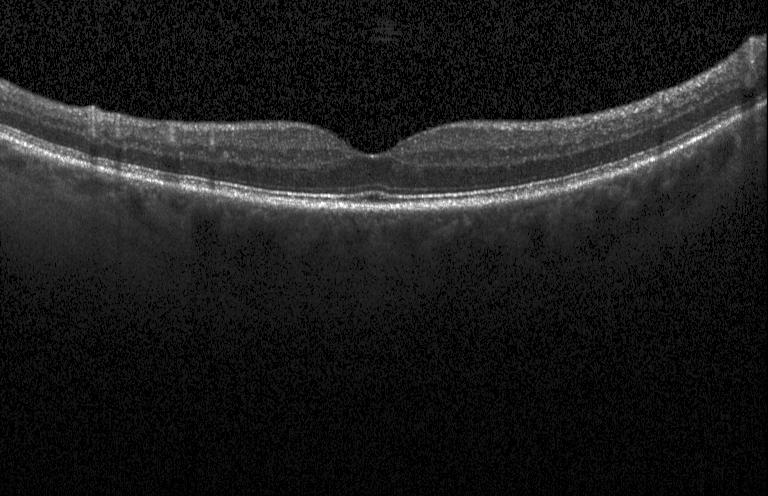
Finding: no choroidal neovascularization, diabetic macular edema, or drusen.